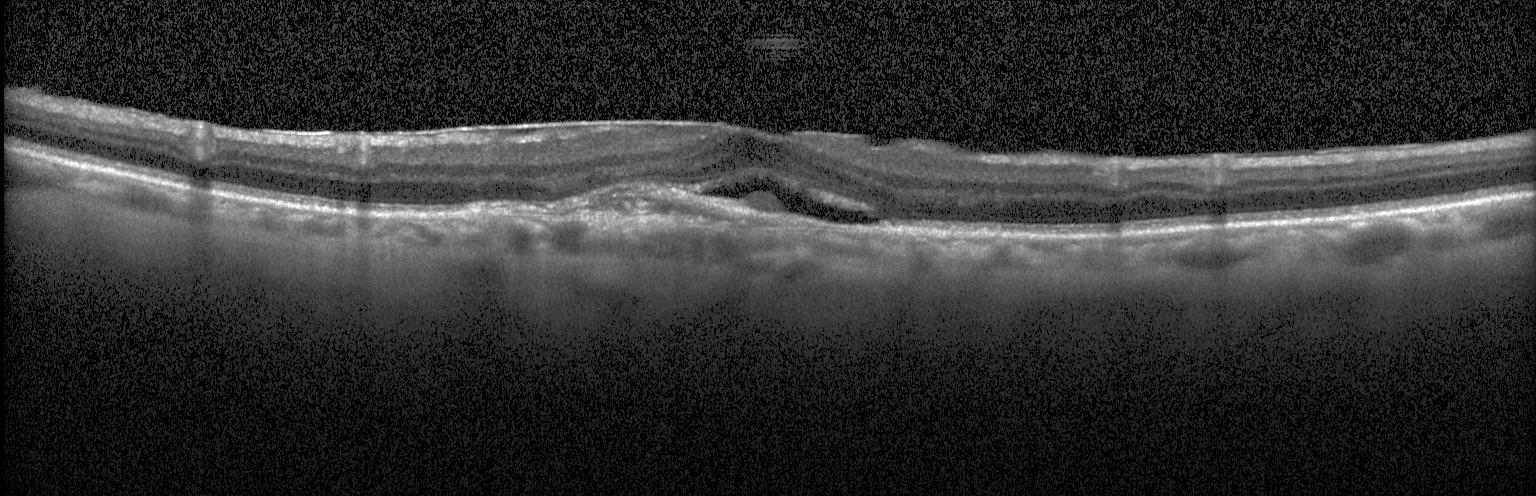 Diagnosis: choroidal neovascularization (CNV).